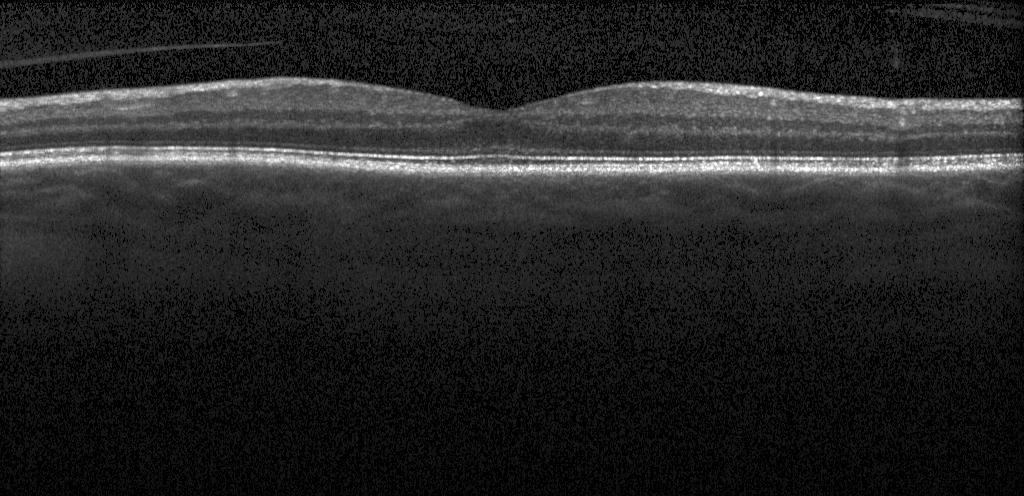
Spectral-domain optical coherence tomography, retinal OCT cross-section.
Dx: neither choroidal neovascularization, diabetic macular edema, nor drusen.